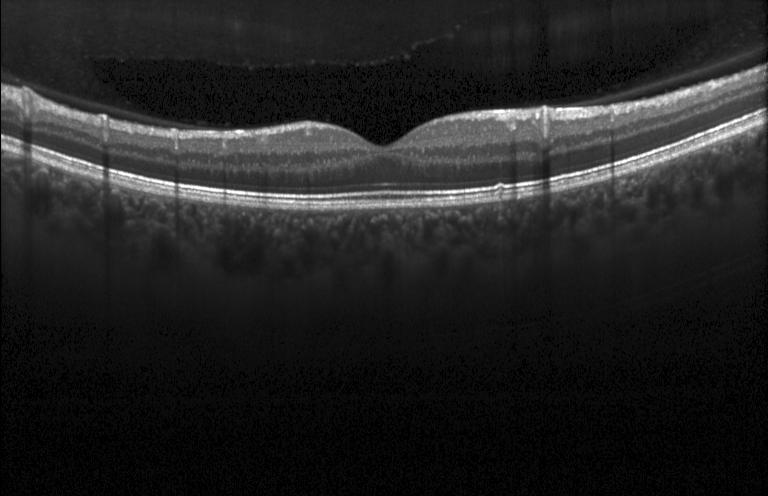
OCT finding: no evidence of choroidal neovascularization, diabetic macular edema, or drusen.